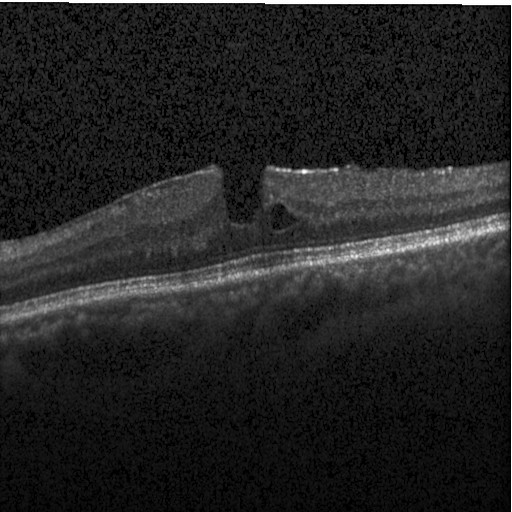
Retinal OCT B-scan. Through the macula.
Diabetic macular edema (DME).